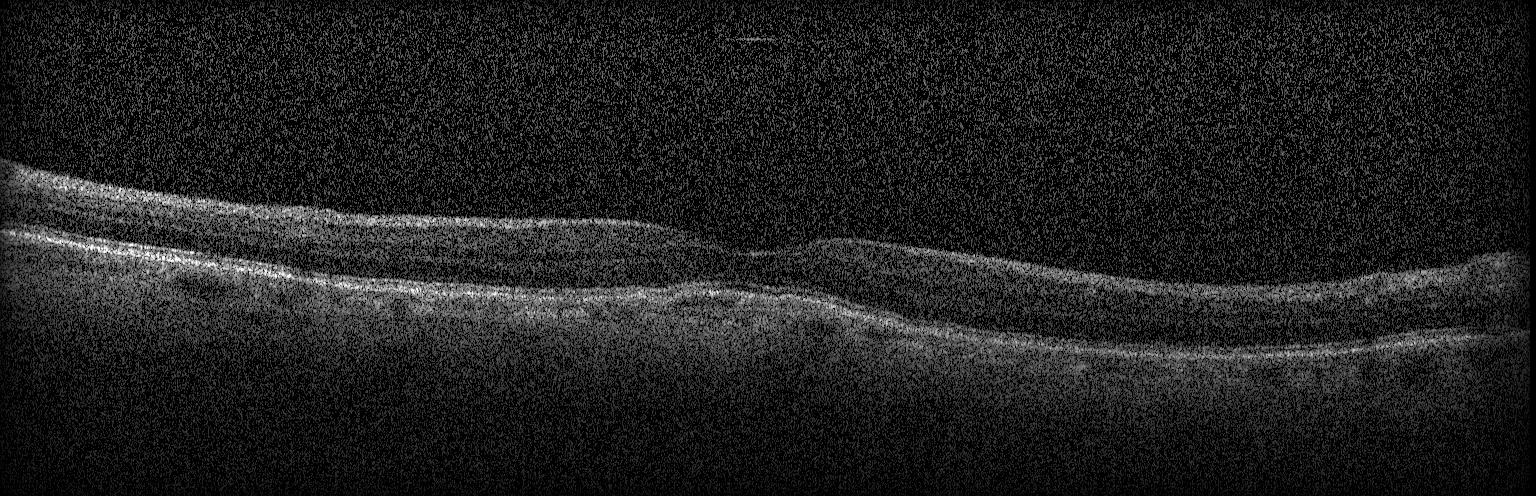 OCT B-scan
Macular OCT: CNV.